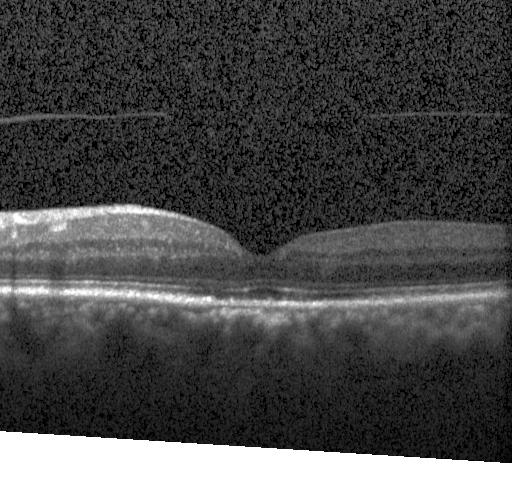

Acquired on a Heidelberg Spectralis; SD-OCT; horizontal scan through the fovea; retinal OCT cross-section.
Impression: no CNV, no DME, and no drusen.